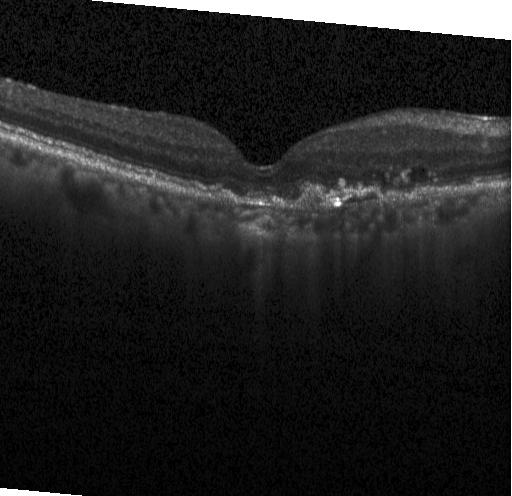
Finding: CNV.